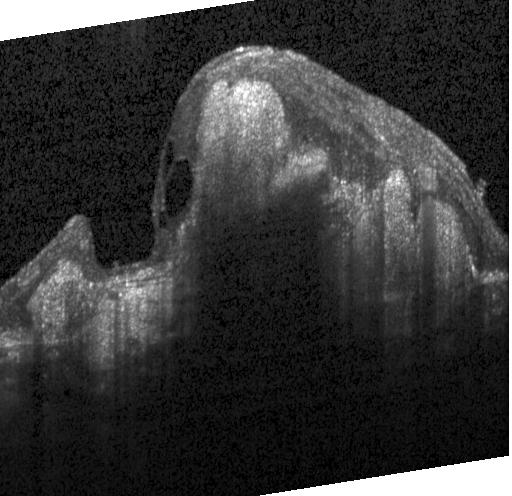 Heidelberg Spectralis, retinal OCT cross-section
Finding: a choroidal neovascular membrane.